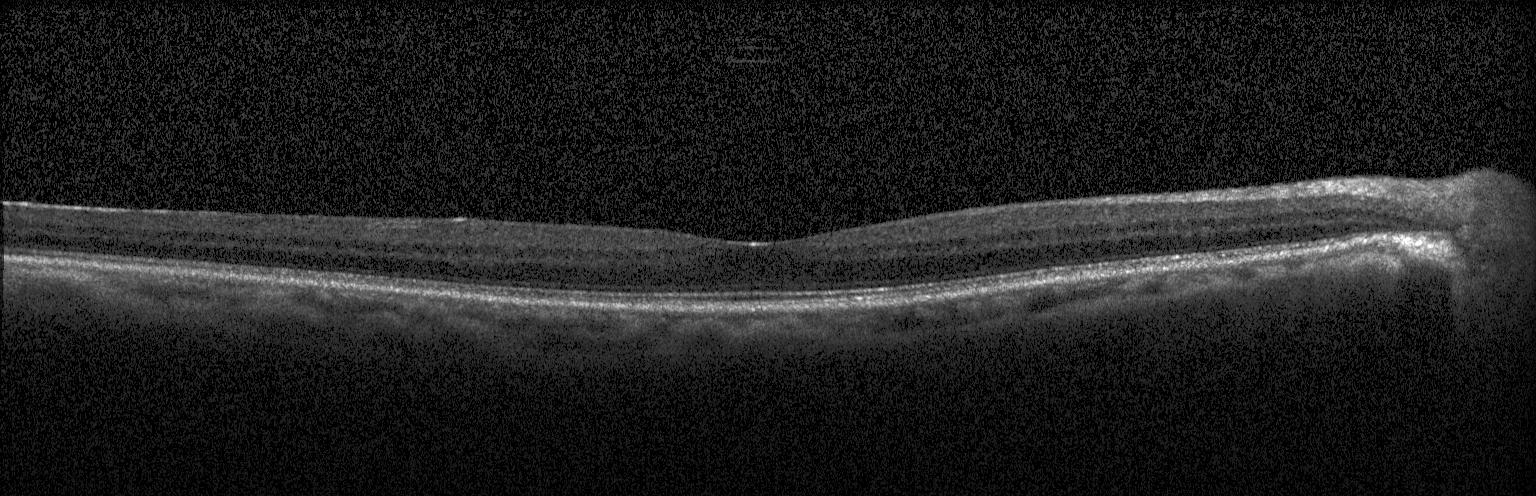

Centered on the fovea, spectral-domain OCT, instrument: Heidelberg Spectralis, retinal OCT B-scan.
Impression: no choroidal neovascularization, no diabetic macular edema, and no drusen.